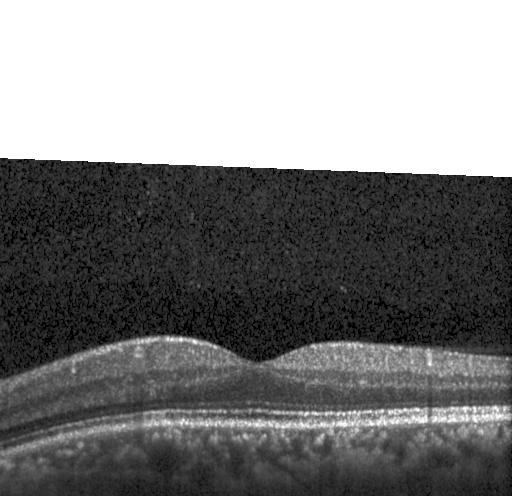
Finding: no evidence of choroidal neovascularization, diabetic macular edema, or drusen.